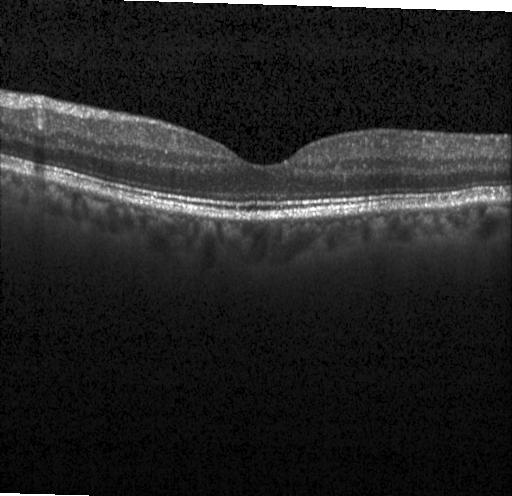

Heidelberg Spectralis; macular scan; OCT line scan; SD-OCT — Diagnosis: no evidence of CNV, DME, or drusen.